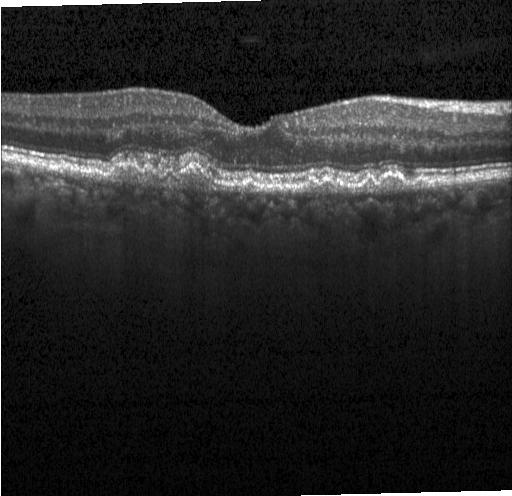
Retinal OCT B-scan — Impression: drusen.